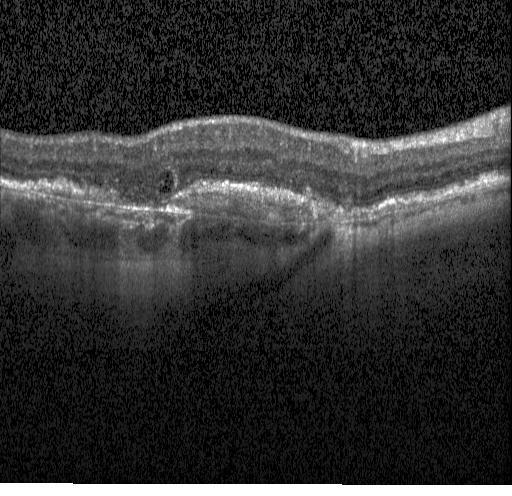 Choroidal neovascularization.